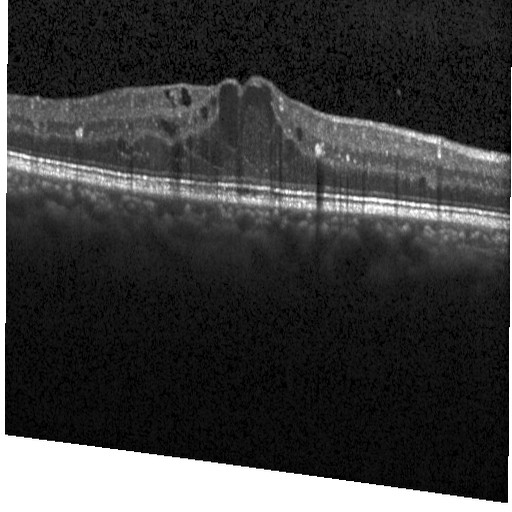

Retinal OCT cross-section showing diabetic macular edema (DME).